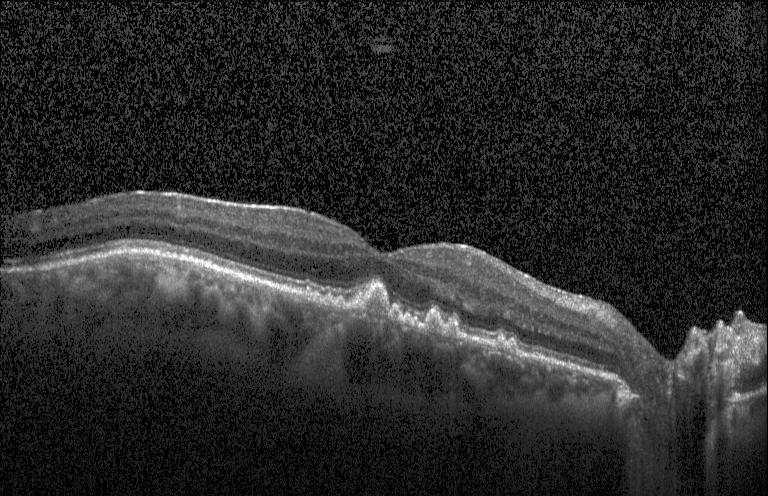
Fovea-centered. Retinal OCT B-scan. Acquired on a Heidelberg Spectralis. Spectral-domain optical coherence tomography — The scan shows drusen.